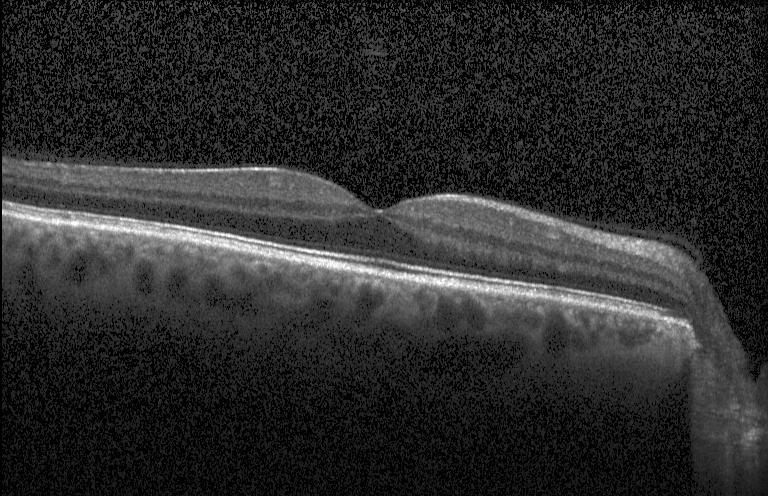

Macular scan · OCT B-scan · instrument: Heidelberg Spectralis
Impression: no evidence of choroidal neovascularization, diabetic macular edema, or drusen.